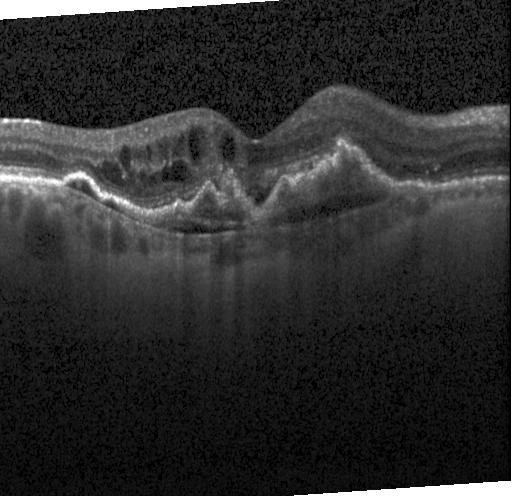
Spectral-domain OCT; macular scan; retinal OCT B-scan
Diagnosis: choroidal neovascularization (CNV).